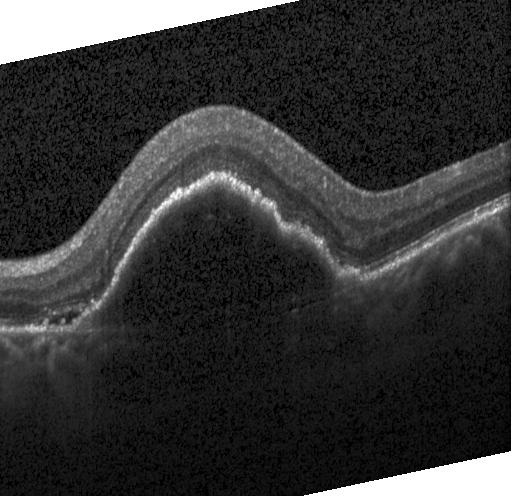 Acquired on a Heidelberg Spectralis, optical coherence tomography scan — Diagnosis: choroidal neovascularization (CNV).